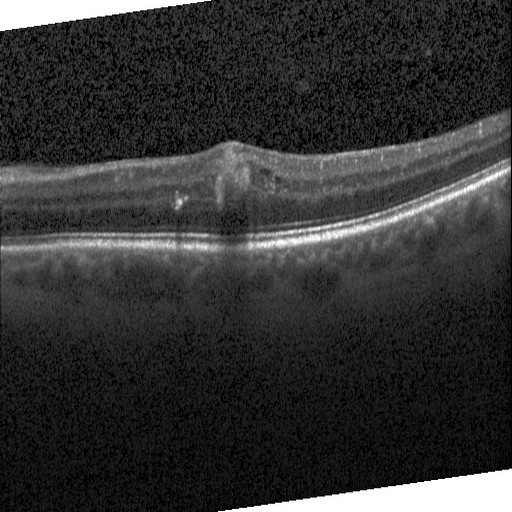 OCT B-scan
Diagnosis: diabetic macular edema (DME).